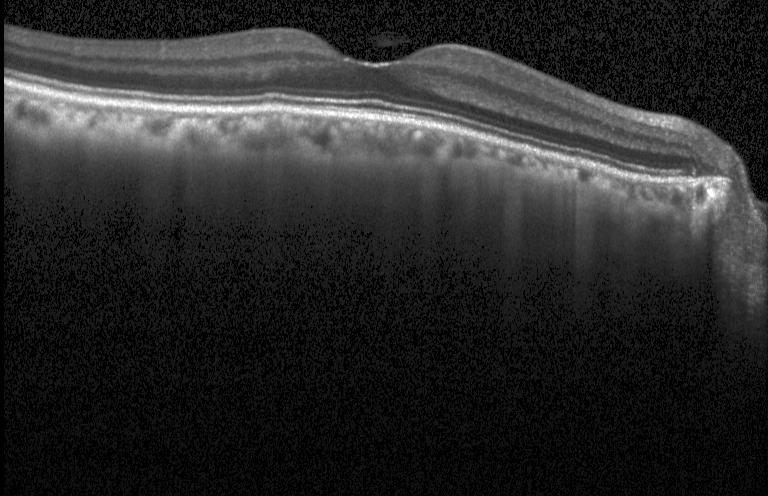 Optical coherence tomography B-scan, horizontal scan through the fovea, Heidelberg Spectralis, SD-OCT — OCT finding: no choroidal neovascularization, no diabetic macular edema, and no drusen.